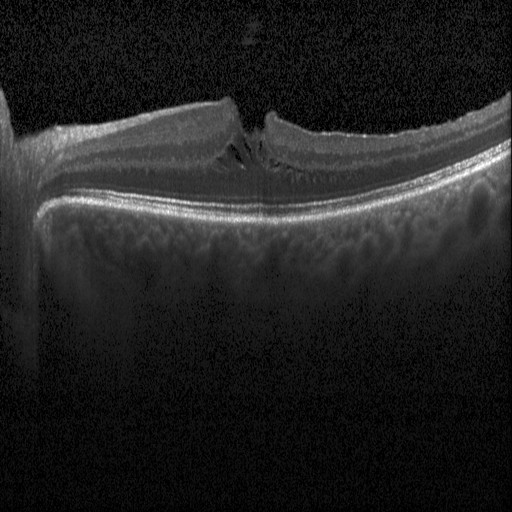
Through the macula. Retinal OCT B-scan. Spectral-domain optical coherence tomography. Finding: diabetic macular edema (DME).